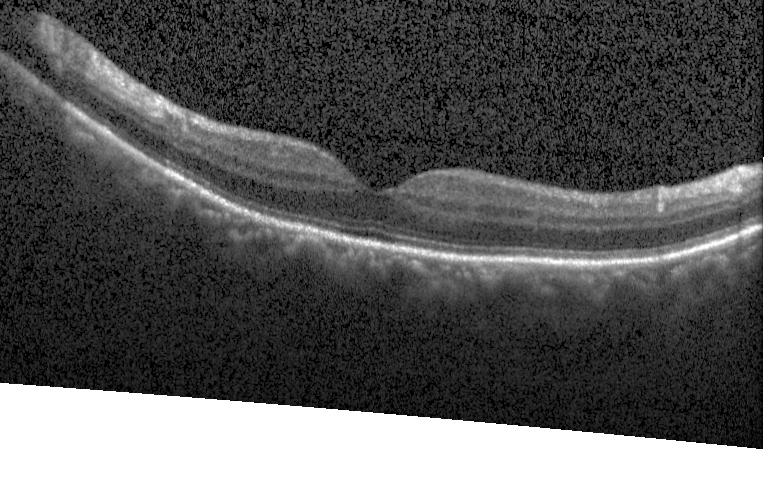
Diagnosis: no choroidal neovascularization, no diabetic macular edema, and no drusen.